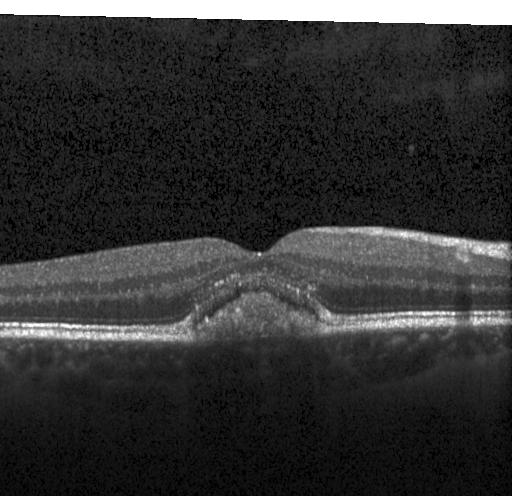
Diagnosis: CNV.